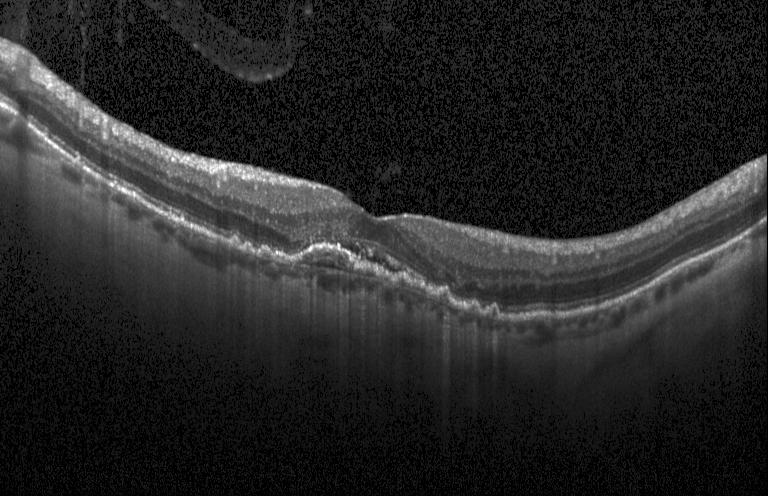
Retinal OCT cross-section showing a choroidal neovascular membrane.